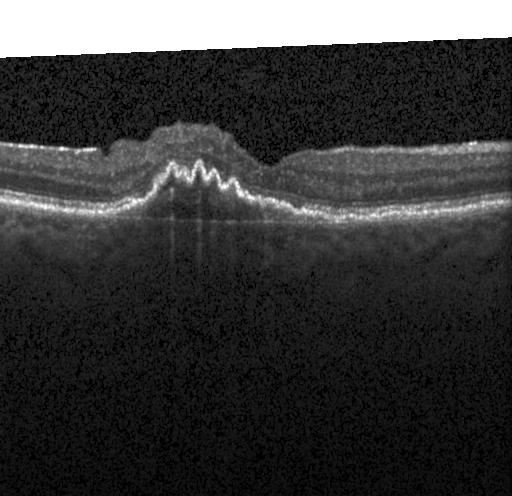

OCT B-scan · Heidelberg Spectralis
The scan shows choroidal neovascularization (CNV).